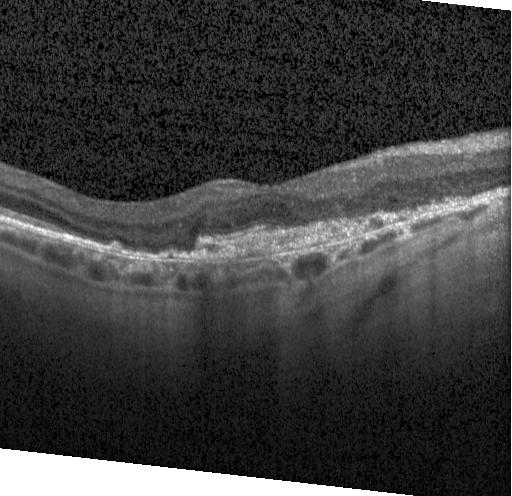

Diagnosis: choroidal neovascularization (CNV).